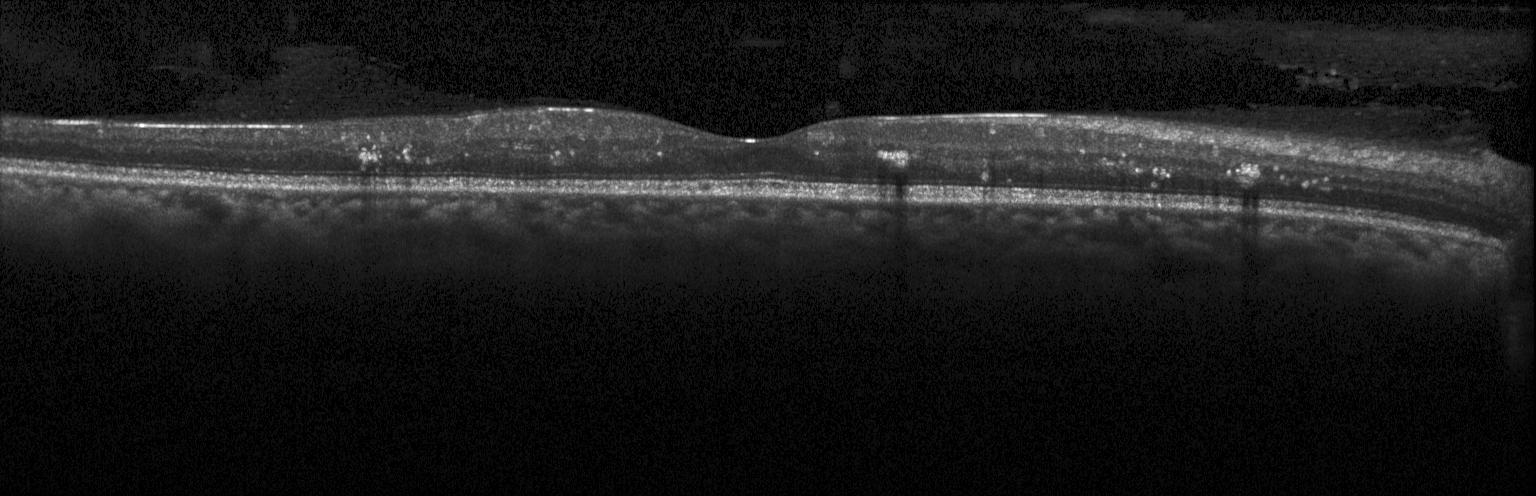 Optical coherence tomography scan, macular scan
The scan shows diabetic macular edema (DME).